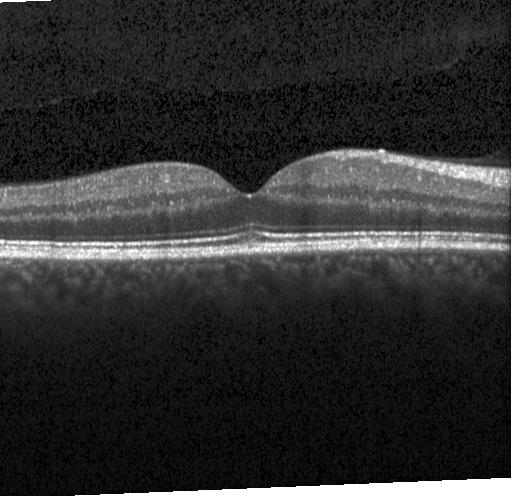

Macular OCT: no choroidal neovascularization, diabetic macular edema, or drusen.